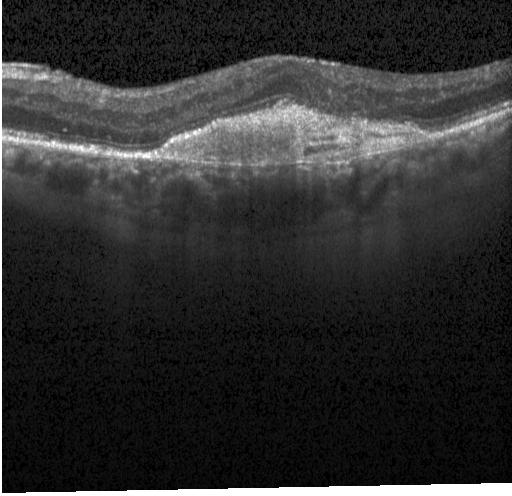
OCT line scan · spectral-domain OCT. OCT finding: choroidal neovascularization (CNV).